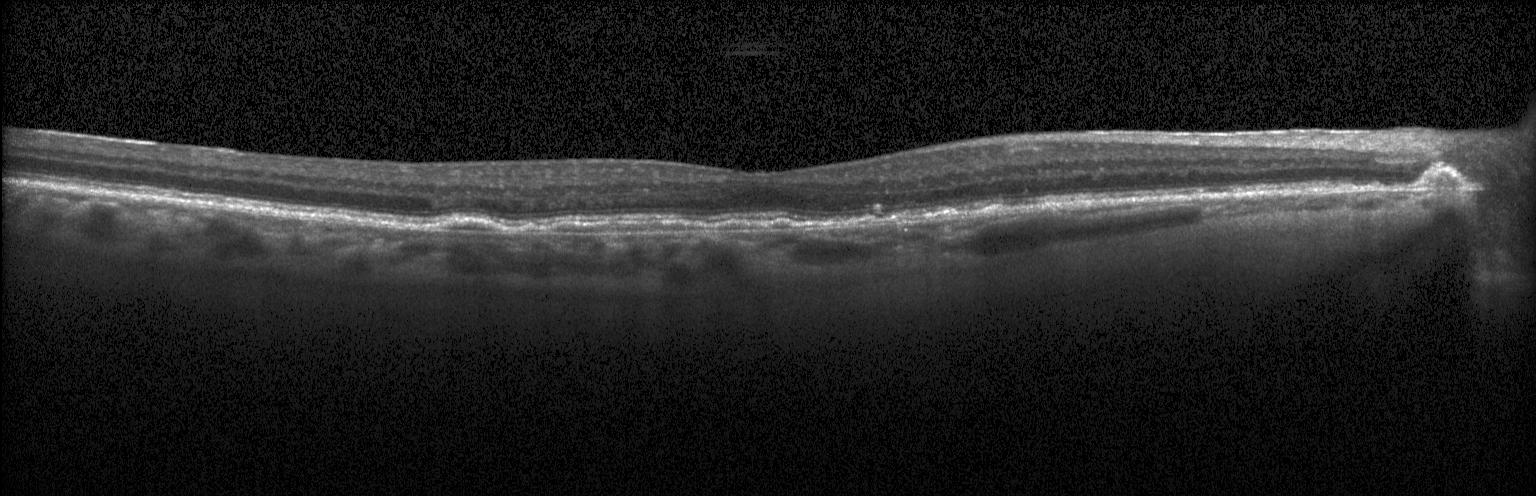
Optical coherence tomography scan, horizontal scan through the fovea
Impression: CNV.